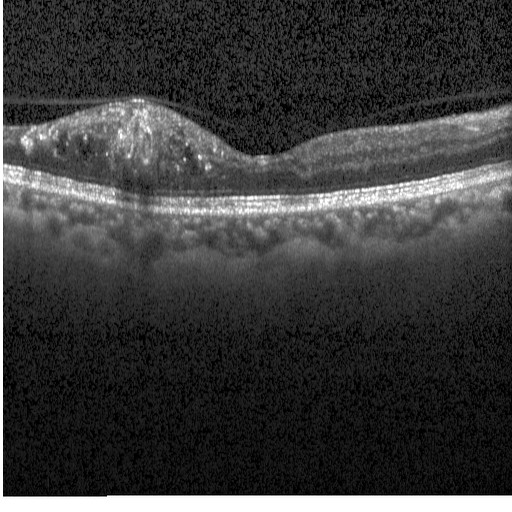 Spectral-domain OCT. OCT line scan. Acquired on a Heidelberg Spectralis
Finding: DME.